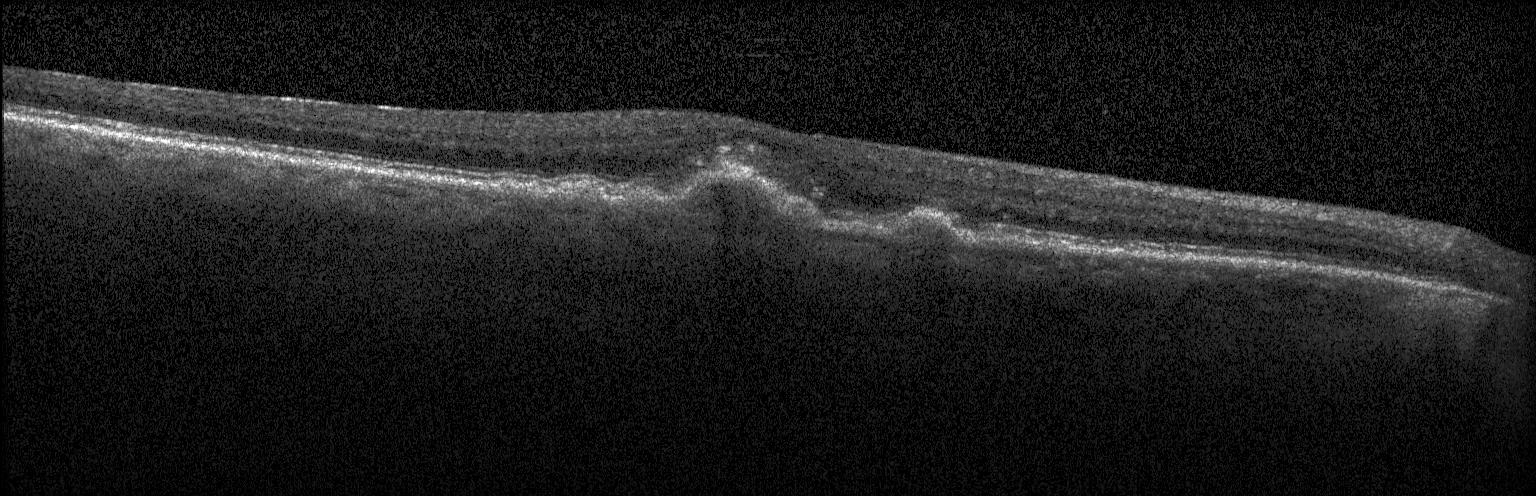
Retinal OCT cross-section. Macular OCT: CNV.